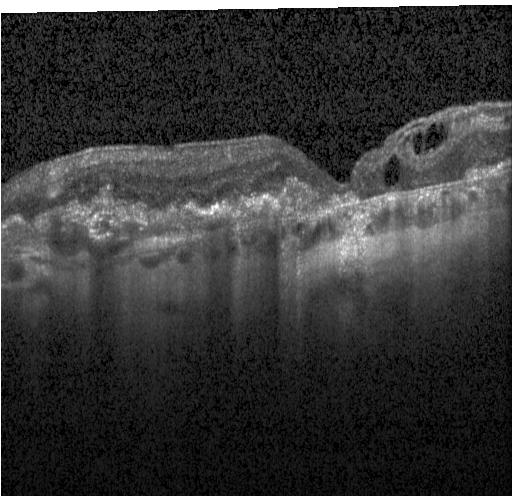

Macular scan · OCT line scan · acquired on a Heidelberg Spectralis
Diagnosis: a choroidal neovascular membrane.